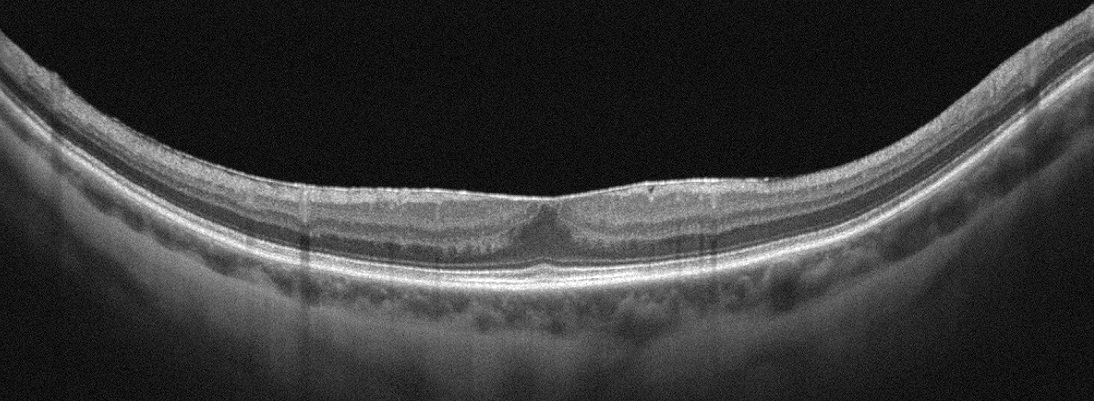

Optovue Avanti RTVue XR; retinal OCT cross-section. Diagnosis: epiretinal membrane (ERM).